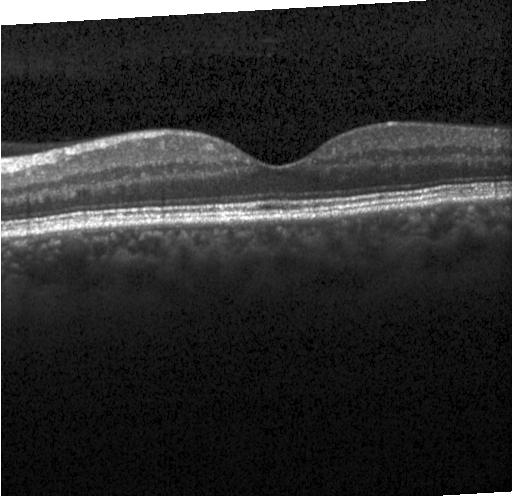 Diagnosis: no choroidal neovascularization, diabetic macular edema, or drusen.